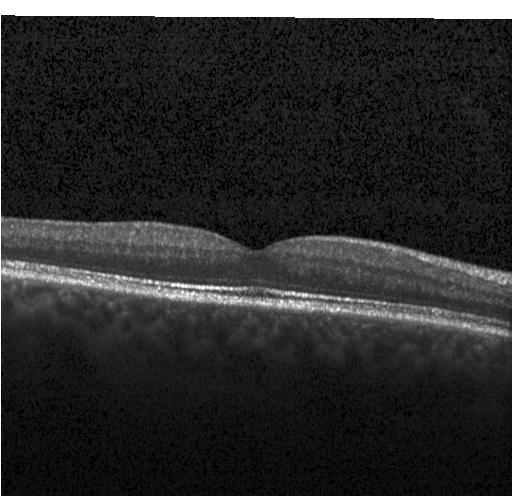

Retinal OCT B-scan.
Impression: no choroidal neovascularization, no diabetic macular edema, and no drusen.